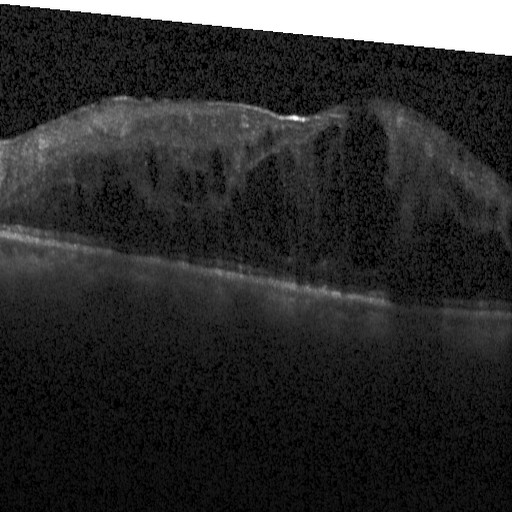 The scan shows diabetic macular edema (DME).